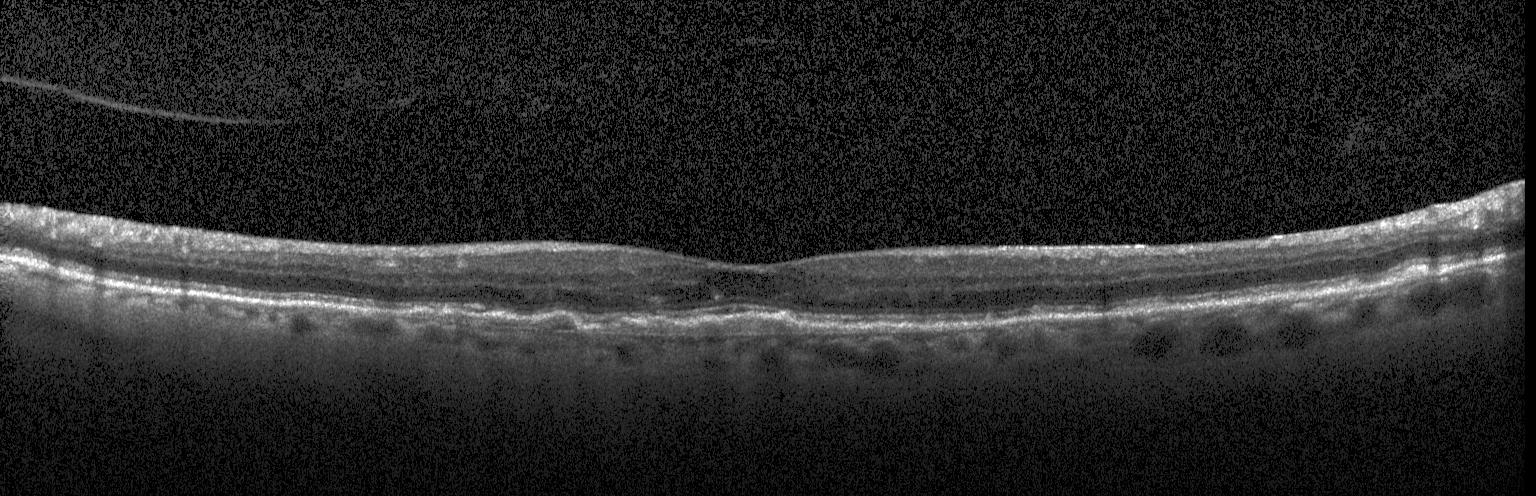

CNV.